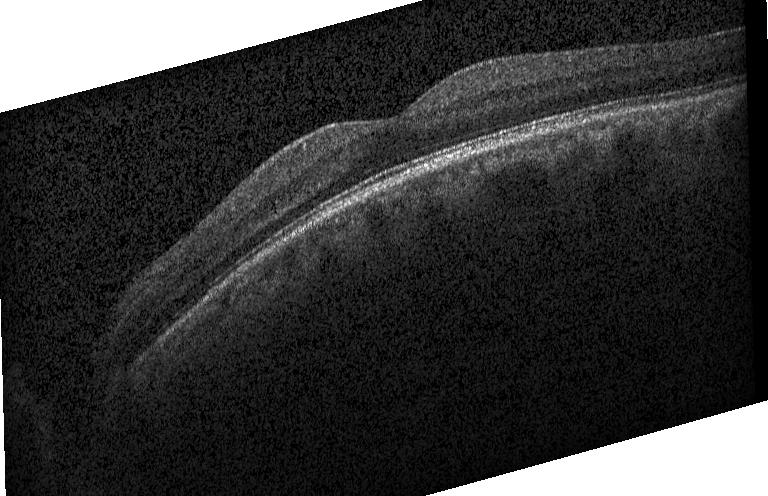 Fovea-centered; spectral-domain optical coherence tomography; optical coherence tomography B-scan; instrument: Heidelberg Spectralis.
Diagnosis: no evidence of CNV, DME, or drusen.